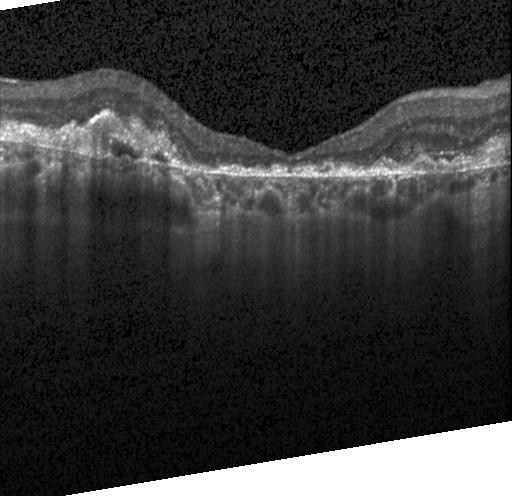

OCT finding: a choroidal neovascular membrane.